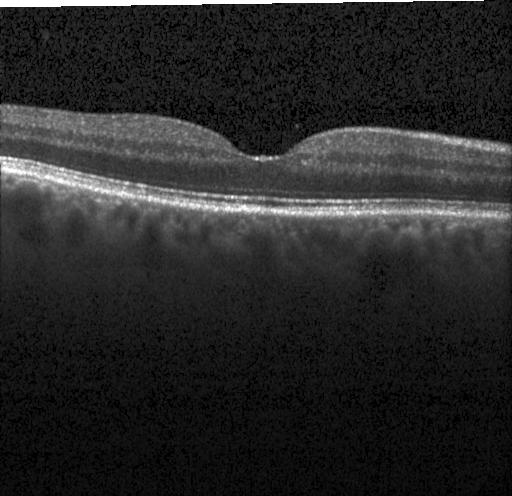 Acquired on a Heidelberg Spectralis, SD-OCT, centered on the fovea, retinal OCT cross-section. Assessment: no CNV, no DME, and no drusen.